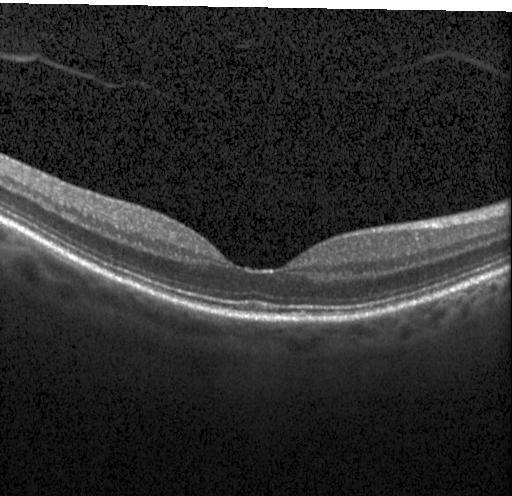

Through the macula · SD-OCT · optical coherence tomography scan · acquired on a Heidelberg Spectralis — Assessment: neither choroidal neovascularization, diabetic macular edema, nor drusen.